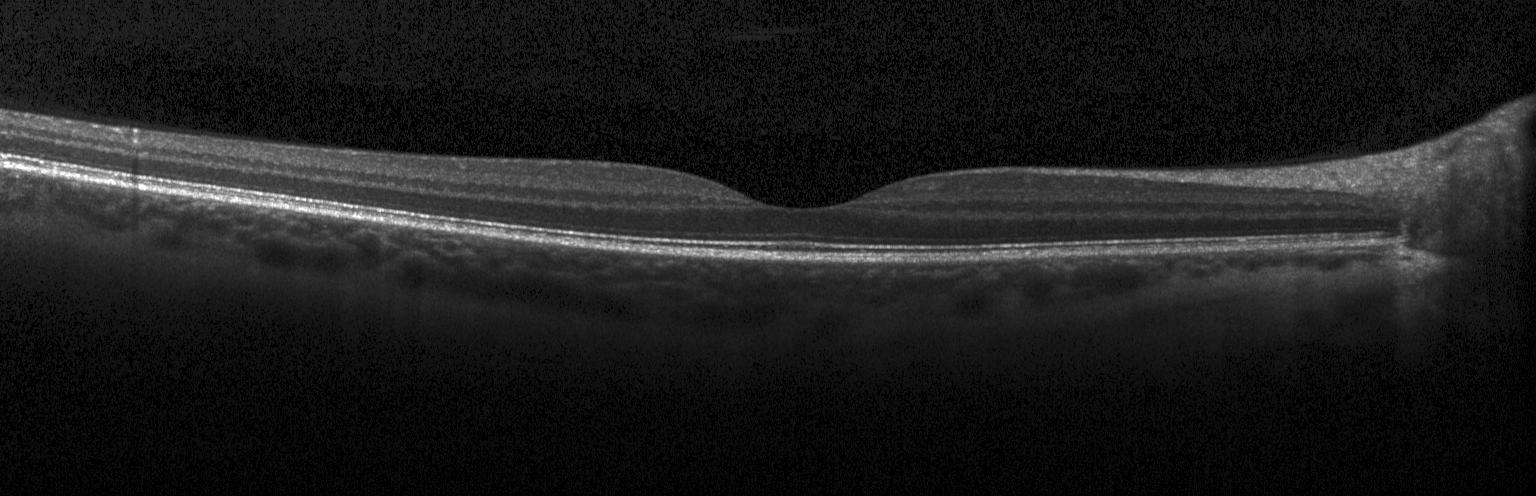

Horizontal scan through the fovea. OCT line scan. The scan shows no CNV, DME, or drusen.